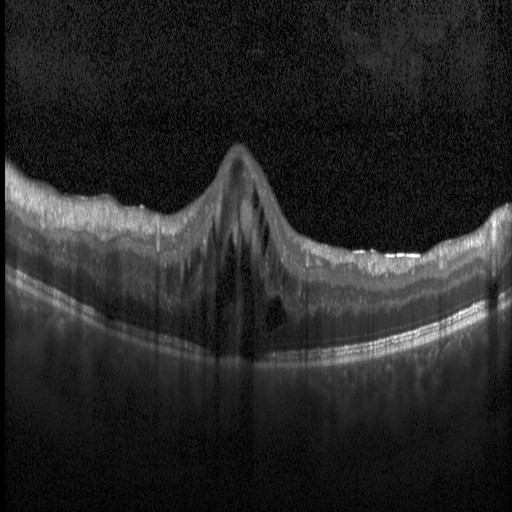
Diabetic macular edema.